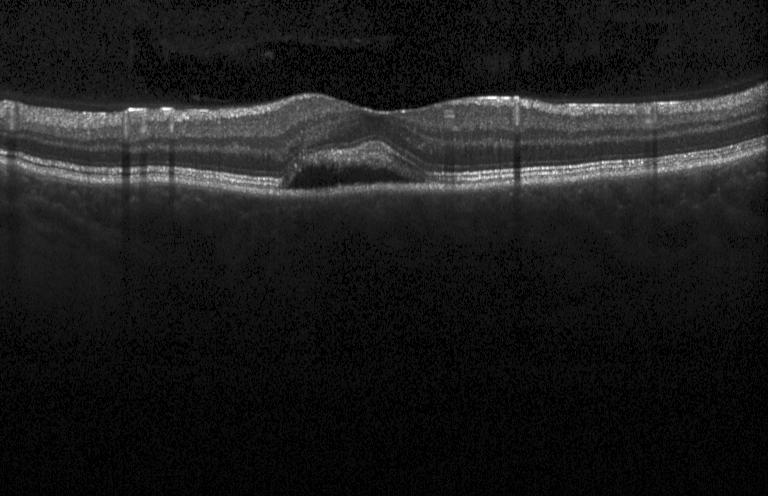

Heidelberg Spectralis OCT system, centered on the fovea, spectral-domain OCT, optical coherence tomography scan.
The scan shows a choroidal neovascular membrane.